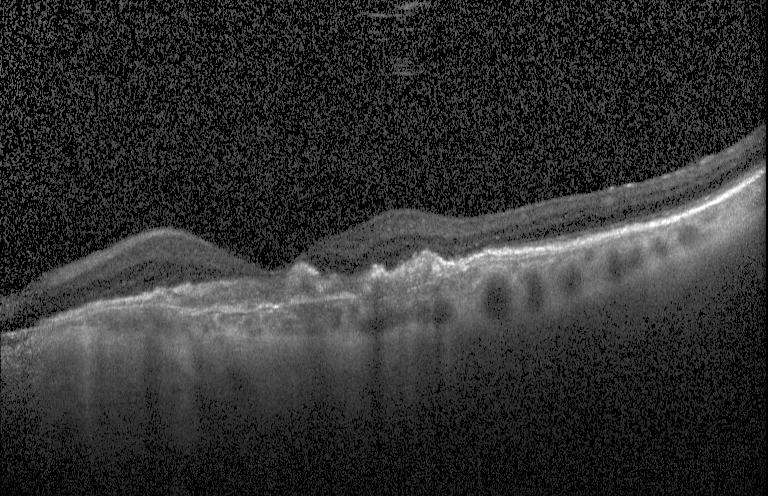

Macular OCT demonstrating a choroidal neovascular membrane.